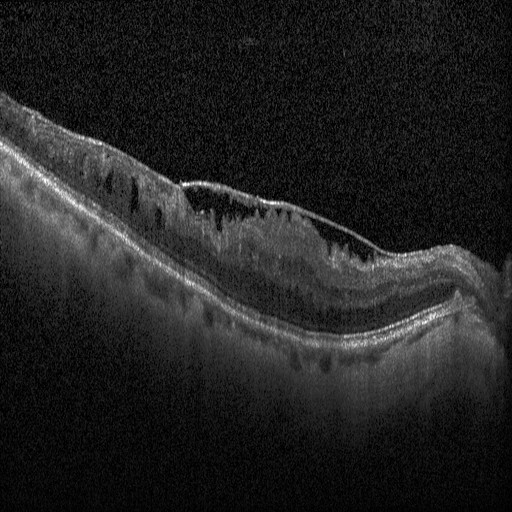
Retinal OCT B-scan.
The scan shows DME.